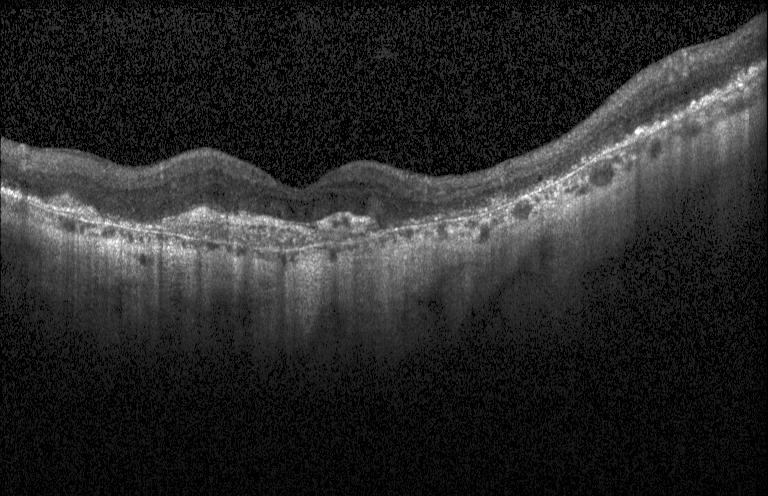
Finding: choroidal neovascularization.